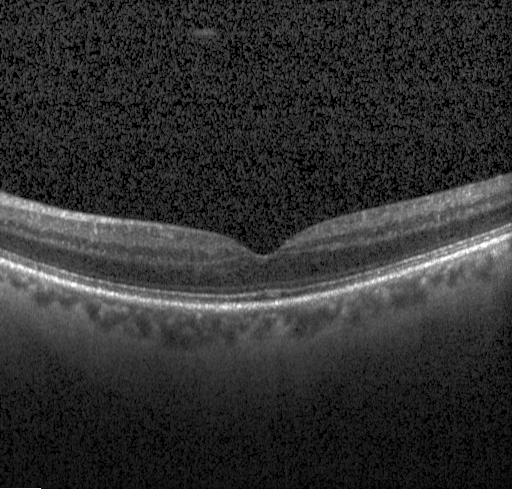

Retinal OCT B-scan; horizontal scan through the fovea; spectral-domain OCT. Impression: no evidence of CNV, DME, or drusen.